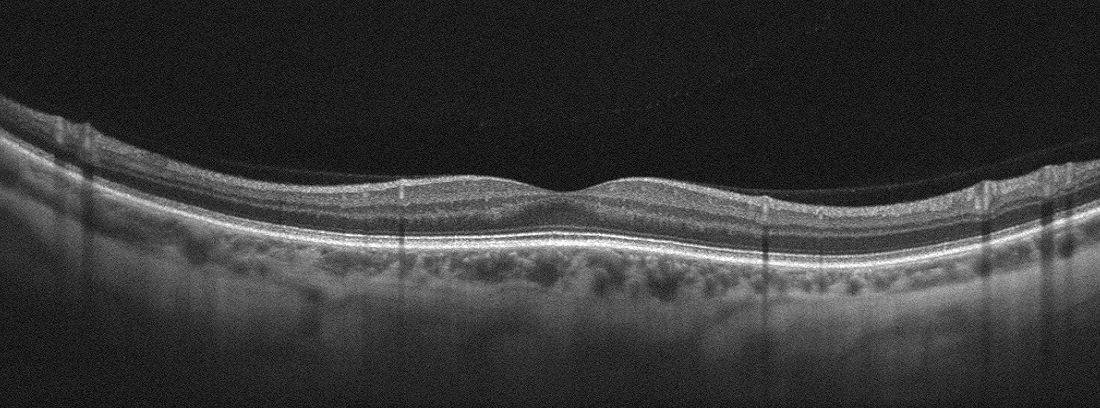 Instrument: Optovue Avanti RTVue XR. Retinal OCT B-scan.
Diagnosis: no evidence of AMD, DME, ERM, RAO, RVO, or VID.